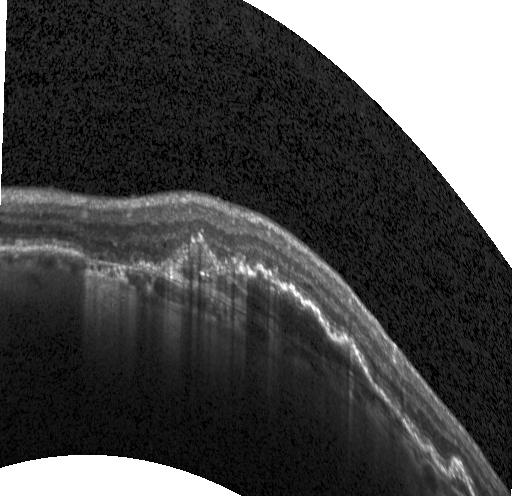 Diagnosis: choroidal neovascularization (CNV).